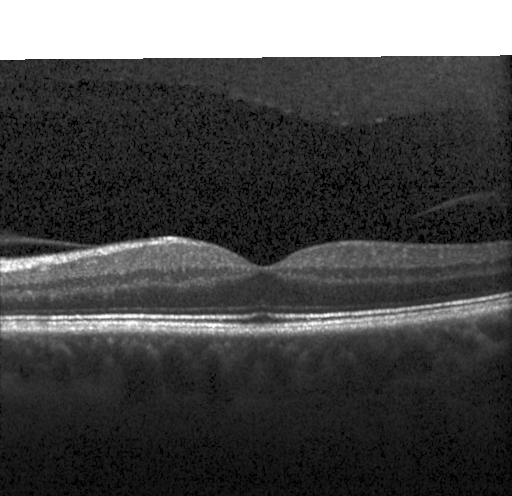
Heidelberg Spectralis OCT system · optical coherence tomography scan · through the macula · SD-OCT — Macular OCT: no choroidal neovascularization, no diabetic macular edema, and no drusen.